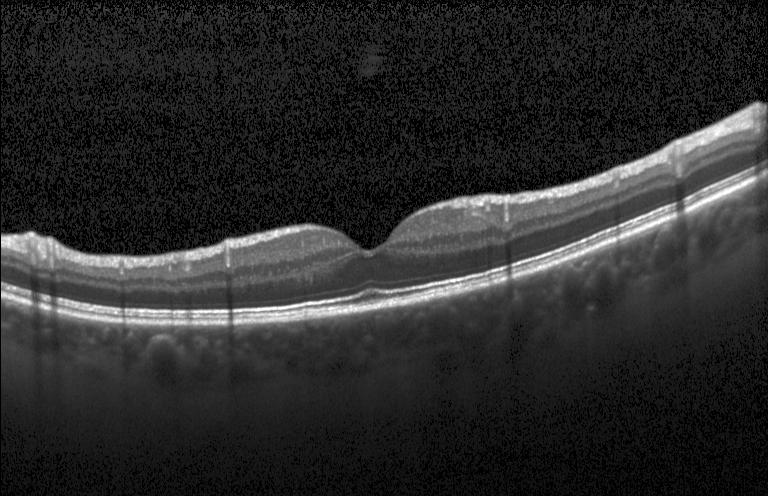 Retinal OCT cross-section showing no evidence of choroidal neovascularization, diabetic macular edema, or drusen.